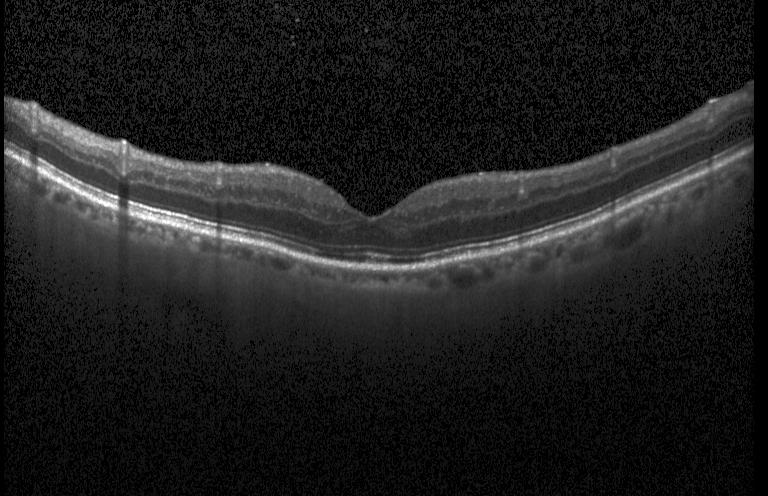
Spectral-domain OCT B-scan: no CNV, DME, or drusen.